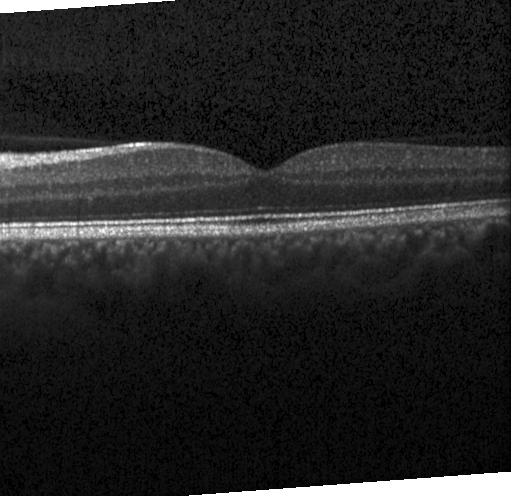 Finding: no CNV, DME, or drusen.